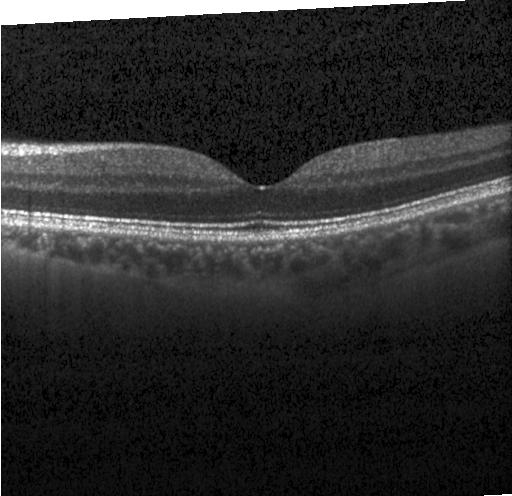 OCT scan showing neither choroidal neovascularization, diabetic macular edema, nor drusen.